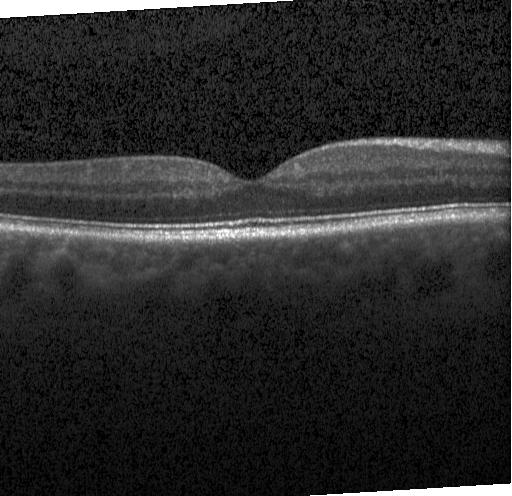
Acquired on a Heidelberg Spectralis · through the macula · optical coherence tomography B-scan · spectral-domain optical coherence tomography.
Assessment: no CNV, no DME, and no drusen.